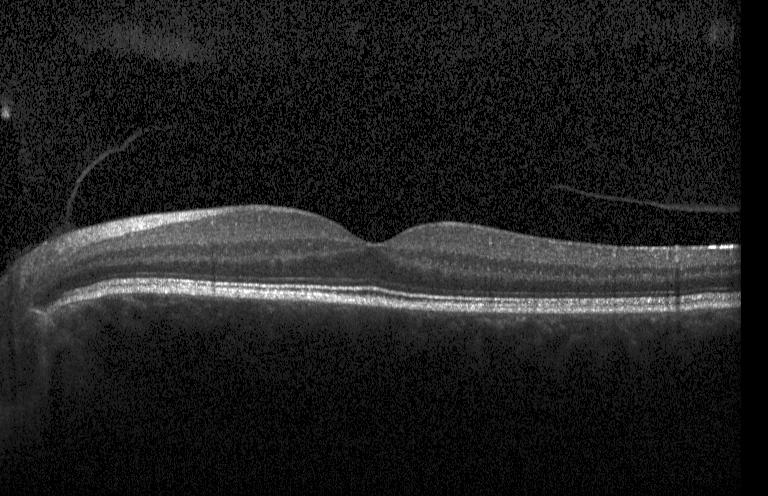 Macular OCT: no choroidal neovascularization, diabetic macular edema, or drusen.